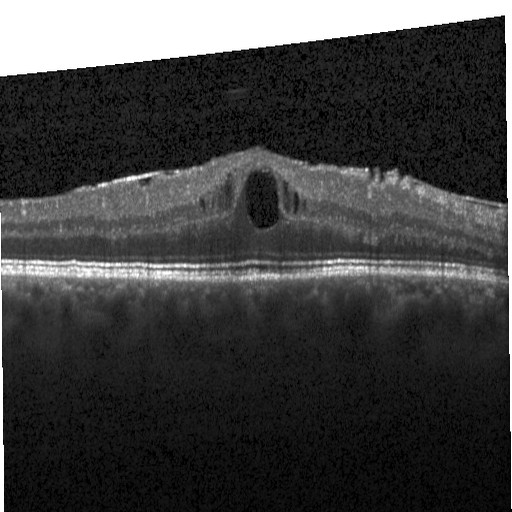

Optical coherence tomography scan · horizontal scan through the fovea · Heidelberg Spectralis
Diagnosis: diabetic macular edema (DME).